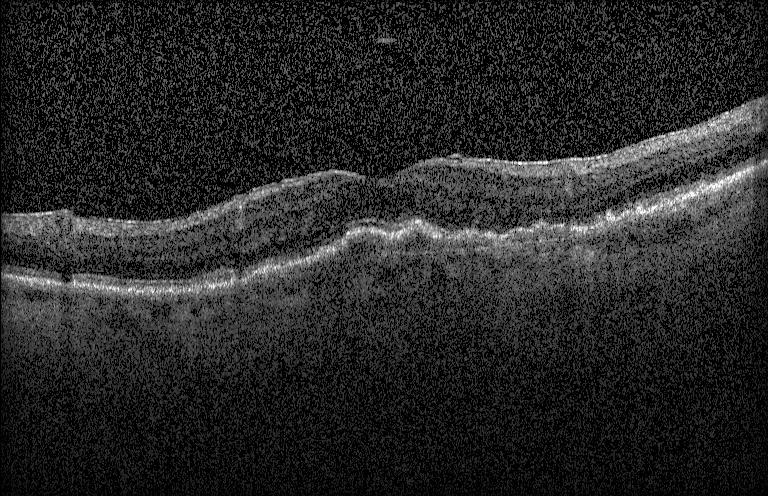 Retinal OCT cross-section.
This B-scan demonstrates choroidal neovascularization.